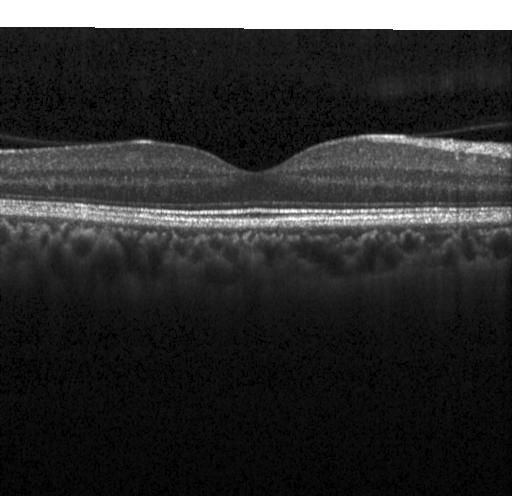

Fovea-centered, acquired on a Heidelberg Spectralis, optical coherence tomography B-scan, SD-OCT. Dx: no evidence of choroidal neovascularization, diabetic macular edema, or drusen.